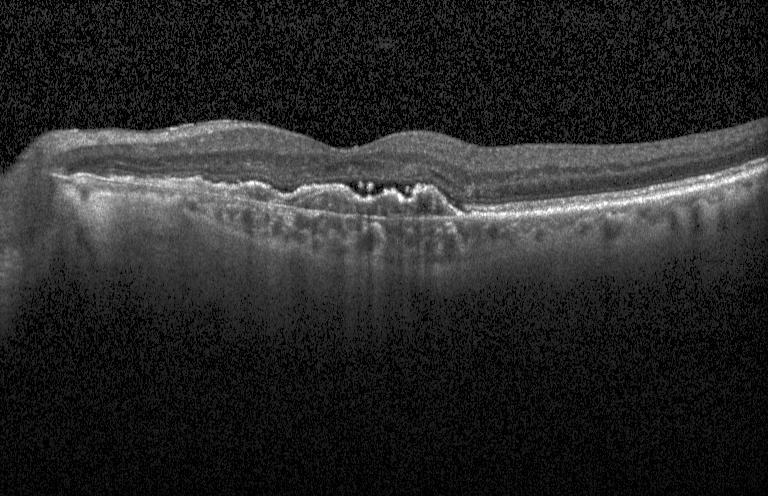

Assessment: choroidal neovascularization (CNV).